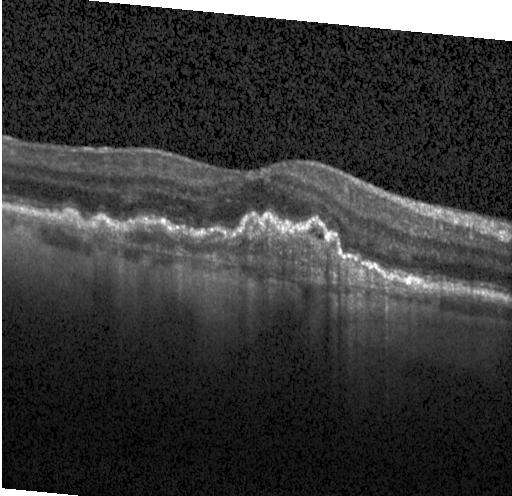
Impression: a choroidal neovascular membrane.